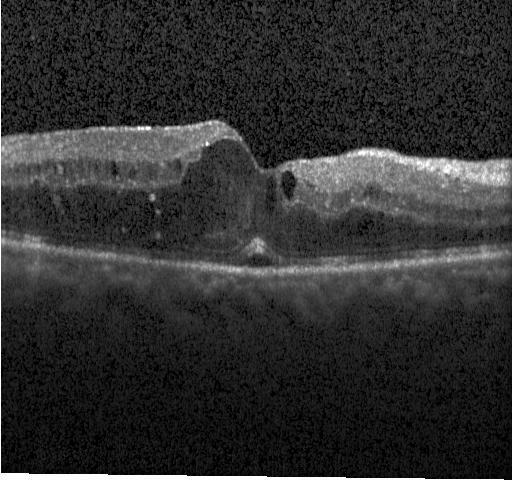 Finding: diabetic macular edema.